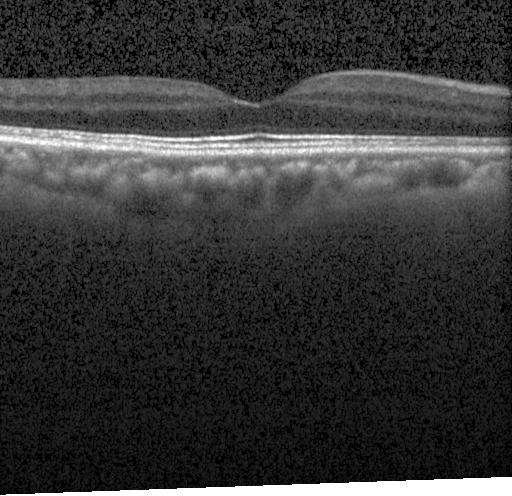
Optical coherence tomography B-scan.
Impression: no evidence of choroidal neovascularization, diabetic macular edema, or drusen.